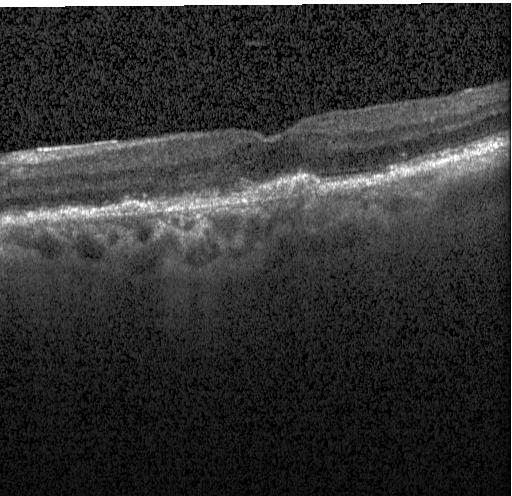 Choroidal neovascularization.